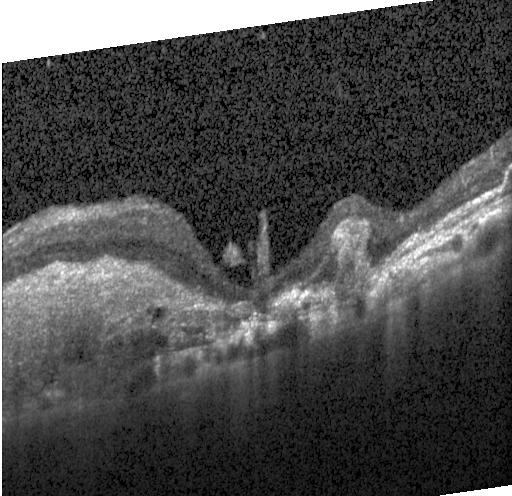 Optical coherence tomography scan · spectral-domain optical coherence tomography · Heidelberg Spectralis · horizontal scan through the fovea. Finding: a choroidal neovascular membrane.